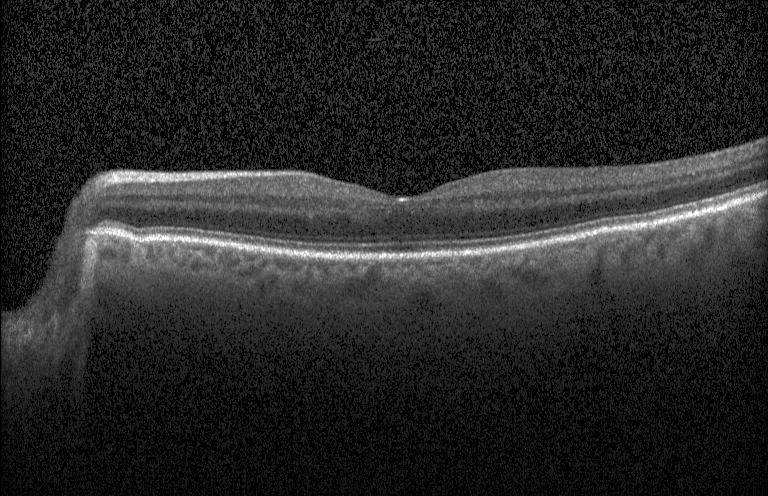
Horizontal scan through the fovea. Optical coherence tomography scan. Acquired on a Heidelberg Spectralis. This B-scan demonstrates no CNV, DME, or drusen.